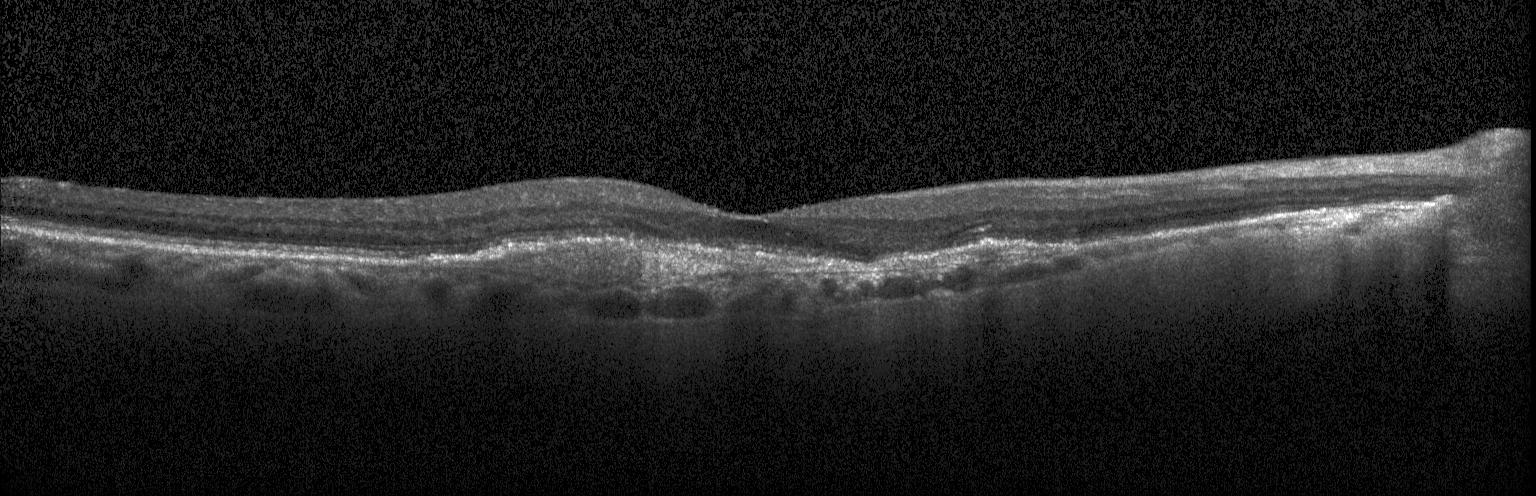

Optical coherence tomography scan; Heidelberg Spectralis; through the macula
Diagnosis: CNV.